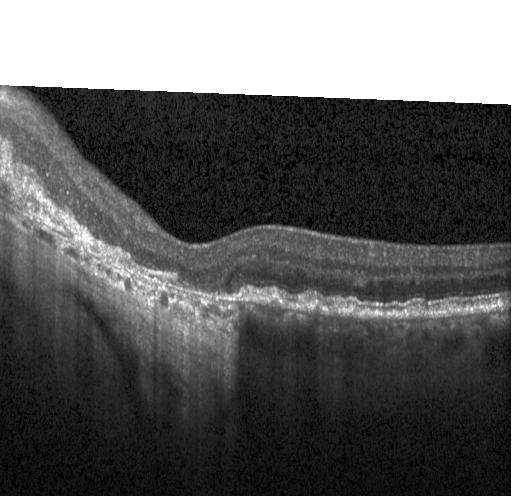 Optical coherence tomography scan. Spectral-domain optical coherence tomography
OCT finding: a choroidal neovascular membrane.